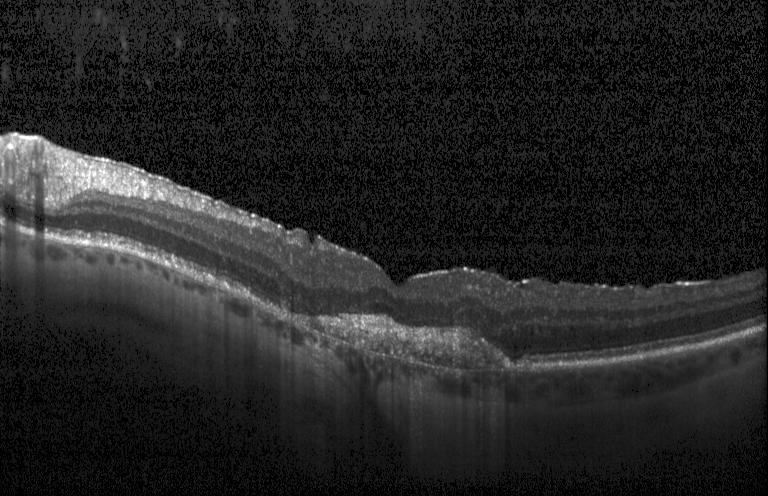

Dx: choroidal neovascularization (CNV).